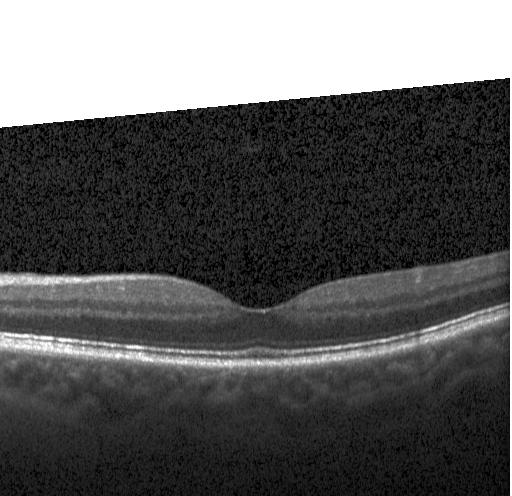

Through the macula. OCT B-scan. Heidelberg Spectralis
Dx: no choroidal neovascularization, no diabetic macular edema, and no drusen.